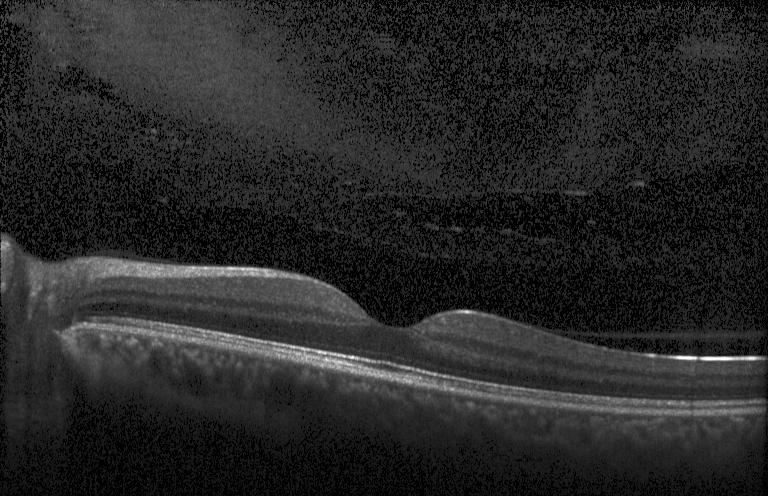

The scan shows no choroidal neovascularization, no diabetic macular edema, and no drusen.